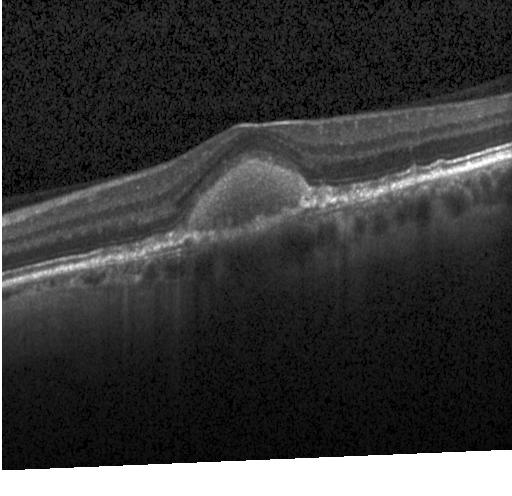

Macular OCT demonstrating choroidal neovascularization (CNV).